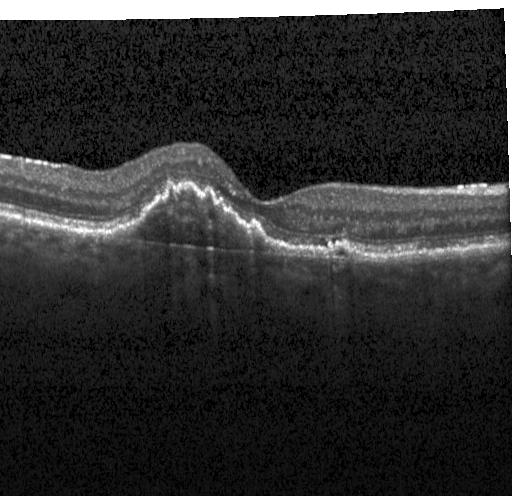
Through the macula; optical coherence tomography scan. Impression: CNV.